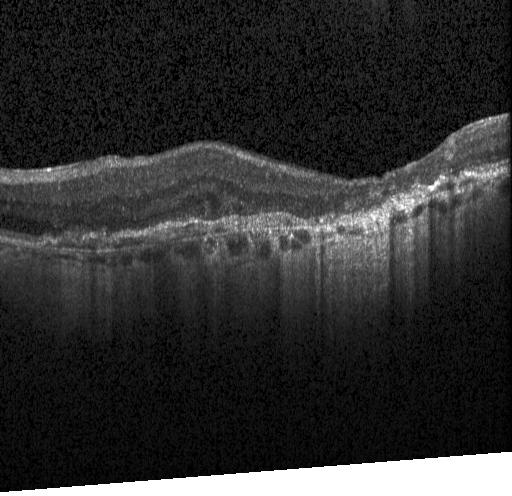
Acquired on a Heidelberg Spectralis. Retinal OCT cross-section
Diagnosis: choroidal neovascularization (CNV).